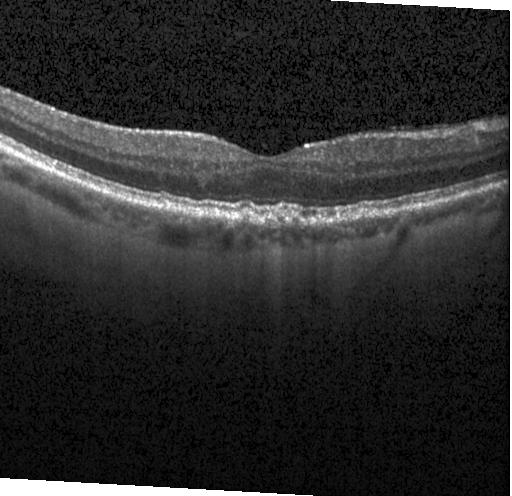 OCT B-scan, spectral-domain OCT, through the macula, Heidelberg Spectralis. Finding: multiple drusen.